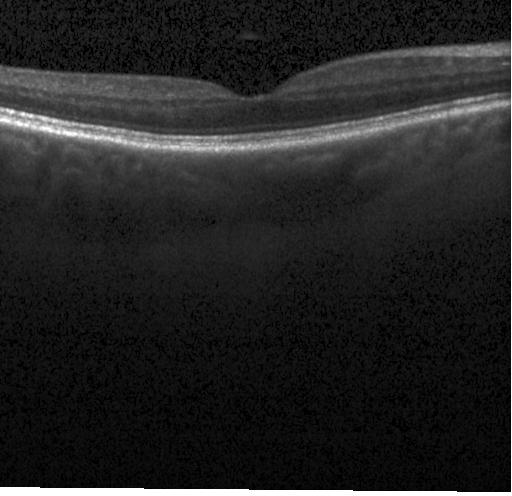

OCT B-scan · spectral-domain OCT · macular scan · Heidelberg Spectralis — Diagnosis: no choroidal neovascularization, diabetic macular edema, or drusen.